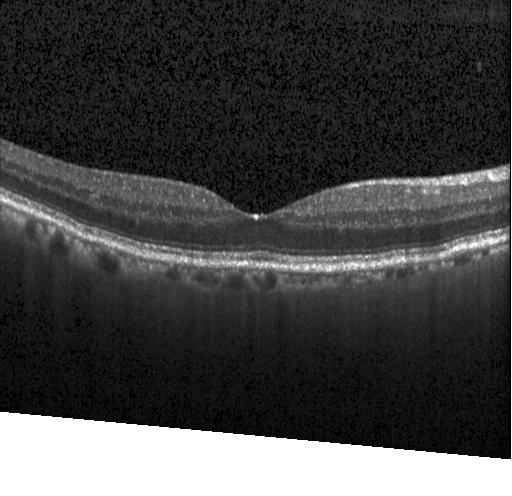
Fovea-centered; Heidelberg Spectralis OCT system; spectral-domain optical coherence tomography; retinal OCT cross-section
No choroidal neovascularization, no diabetic macular edema, and no drusen.